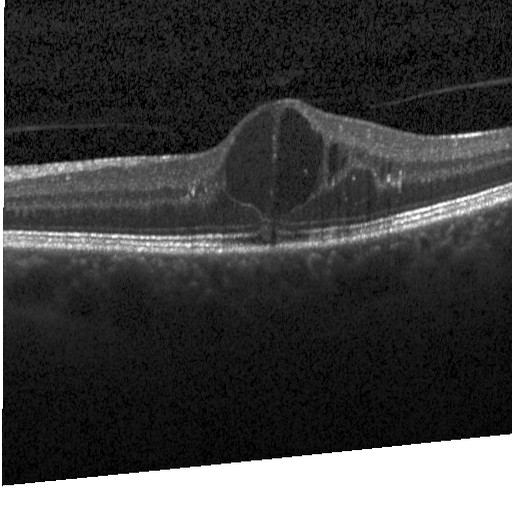
Optical coherence tomography scan — OCT finding: diabetic macular edema (DME).